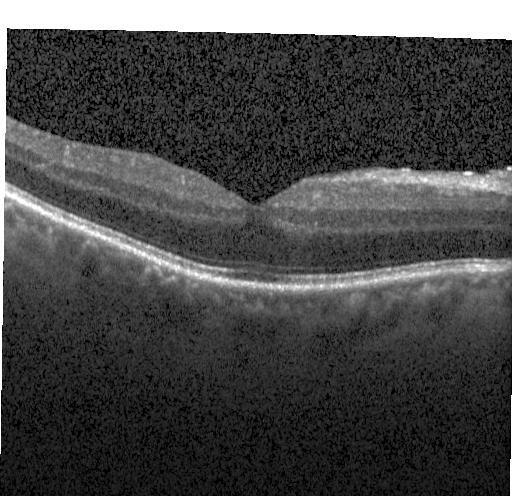 Instrument: Heidelberg Spectralis; centered on the fovea; spectral-domain OCT; optical coherence tomography B-scan. Assessment: no choroidal neovascularization, diabetic macular edema, or drusen.